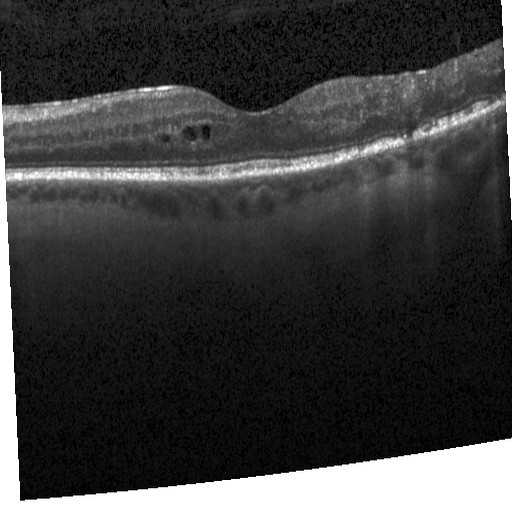 Instrument: Heidelberg Spectralis; spectral-domain OCT; retinal OCT cross-section; through the macula.
Diagnosis: DME.